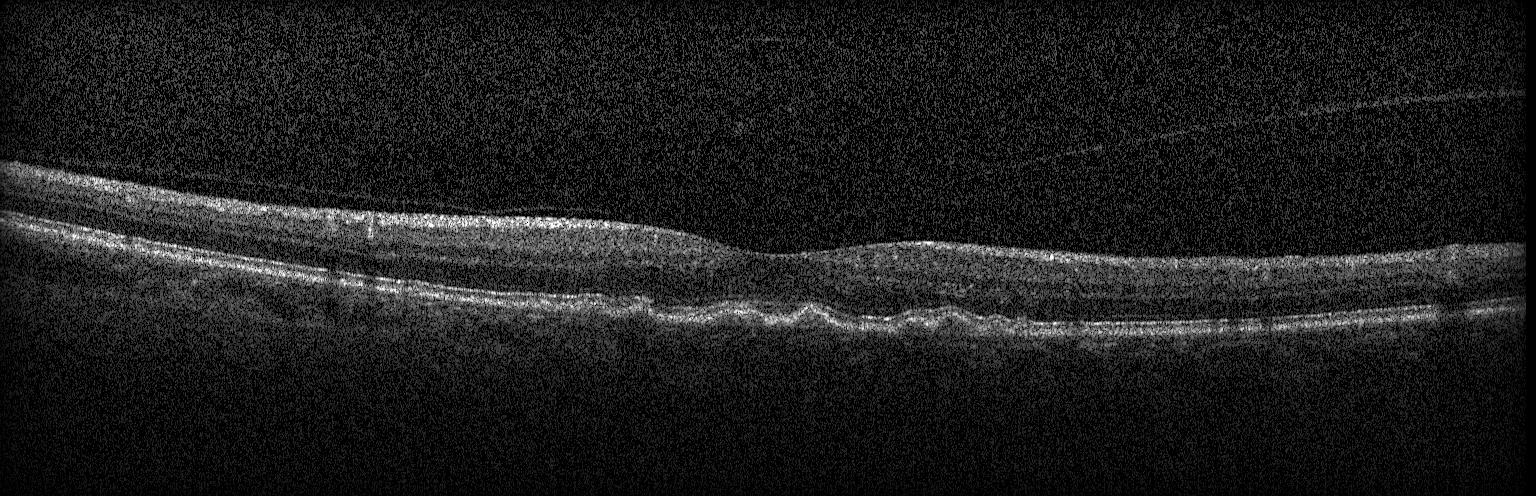 Retinal OCT cross-section. Diagnosis: multiple drusen.